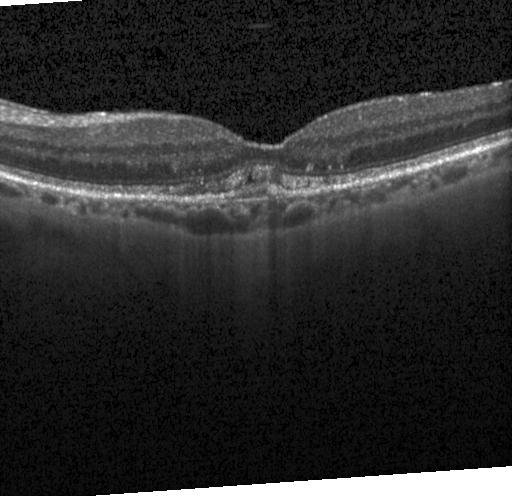 Finding: a choroidal neovascular membrane.